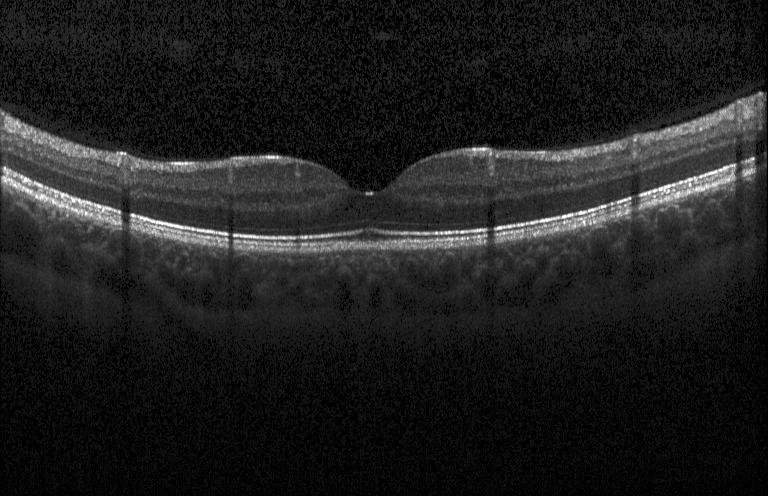
Optical coherence tomography scan, Heidelberg Spectralis, spectral-domain optical coherence tomography
Finding: no evidence of CNV, DME, or drusen.